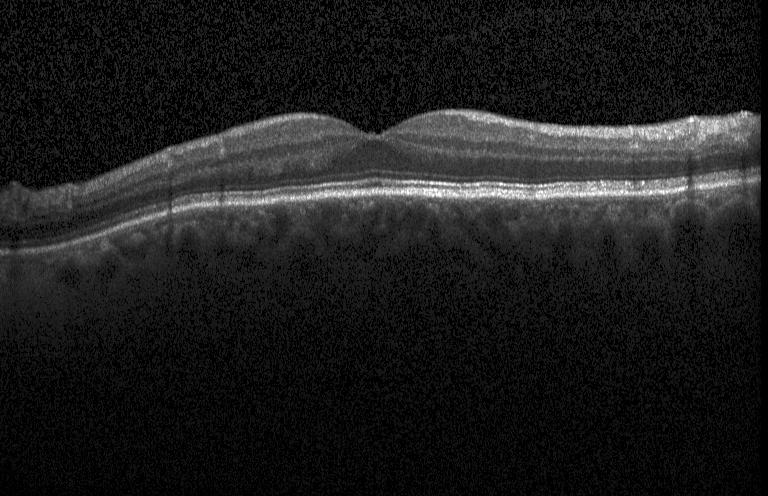 Finding: no choroidal neovascularization, diabetic macular edema, or drusen.